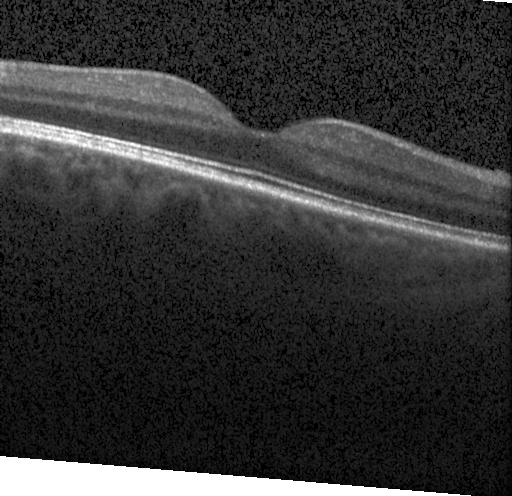

Optical coherence tomography B-scan. Heidelberg Spectralis — OCT finding: no choroidal neovascularization, no diabetic macular edema, and no drusen.